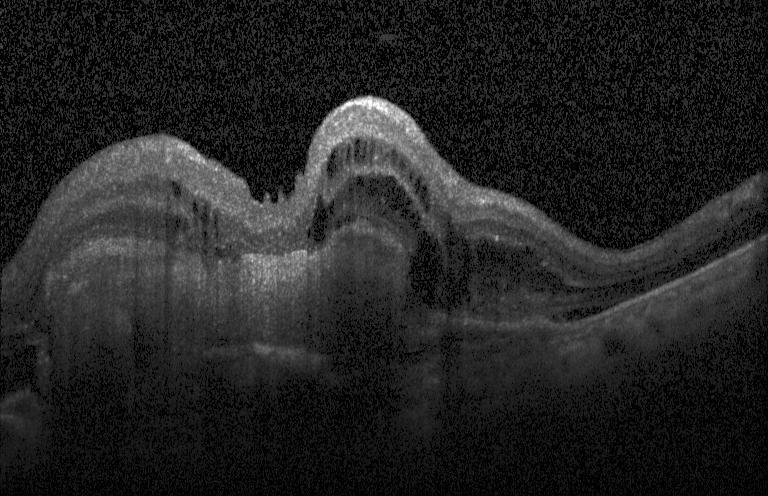 Macular OCT demonstrating a choroidal neovascular membrane.